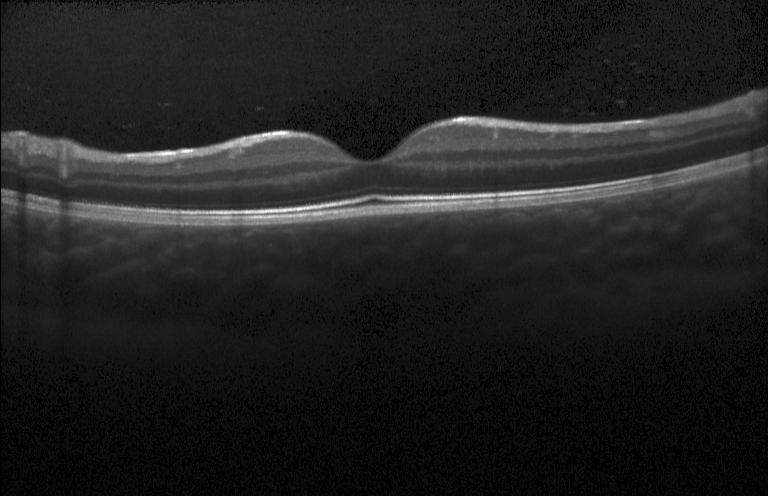 Optical coherence tomography B-scan. Macular OCT: no choroidal neovascularization, diabetic macular edema, or drusen.